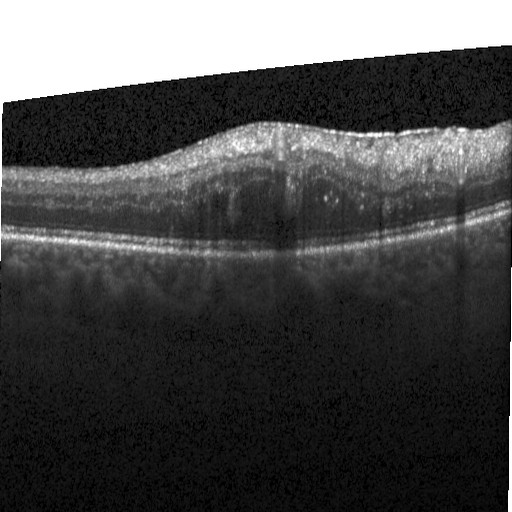
Optical coherence tomography scan
Finding: DME.